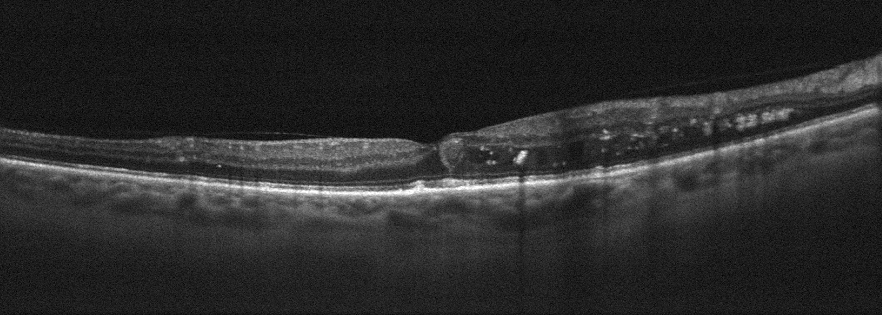 Dx: DME.